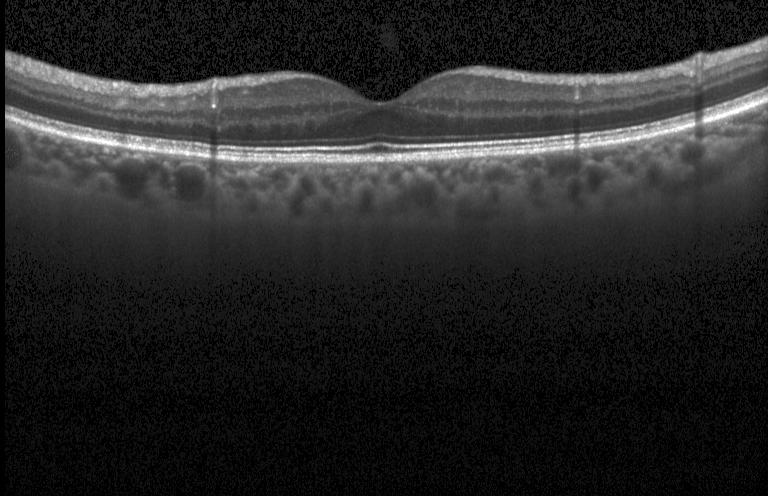
Optical coherence tomography B-scan. Impression: no CNV, DME, or drusen.